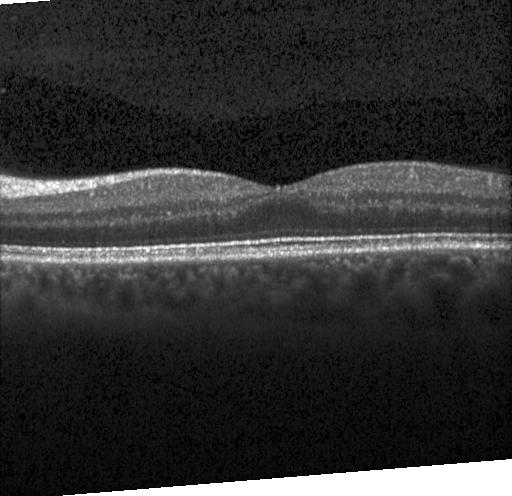

OCT B-scan showing neither choroidal neovascularization, diabetic macular edema, nor drusen.